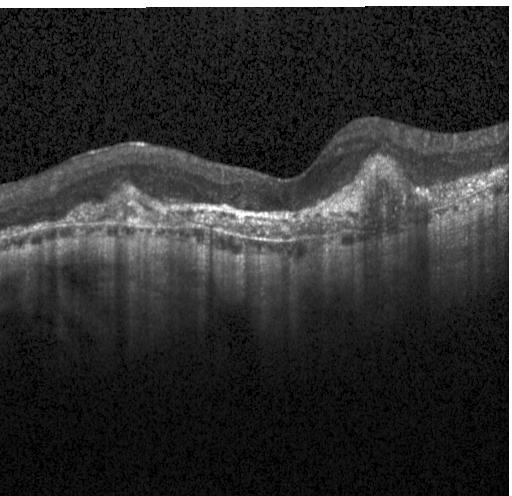
OCT B-scan, Heidelberg Spectralis OCT system, spectral-domain OCT.
Finding: a choroidal neovascular membrane.